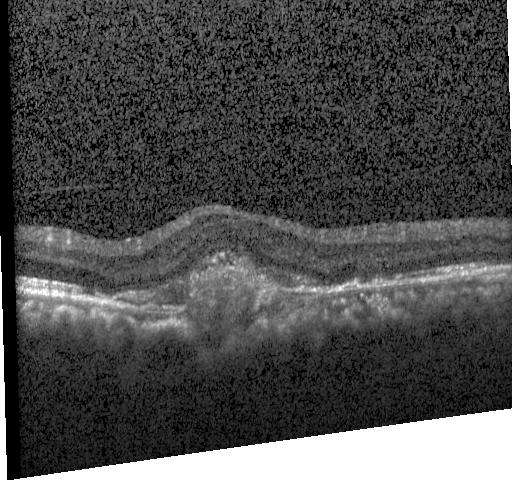 Finding: CNV.